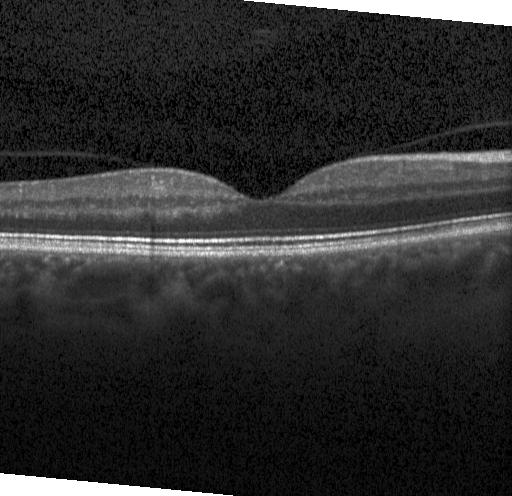
OCT B-scan. SD-OCT. Heidelberg Spectralis. Horizontal scan through the fovea — Impression: no choroidal neovascularization, diabetic macular edema, or drusen.